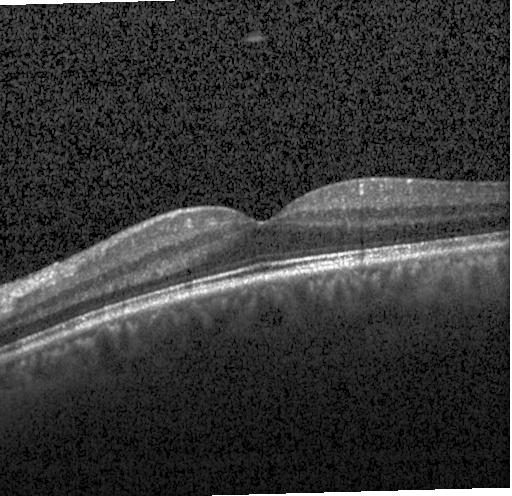
Diagnosis: no choroidal neovascularization, diabetic macular edema, or drusen.